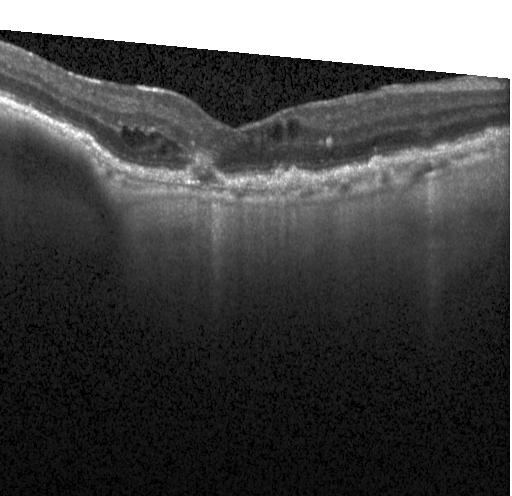
Assessment: CNV.